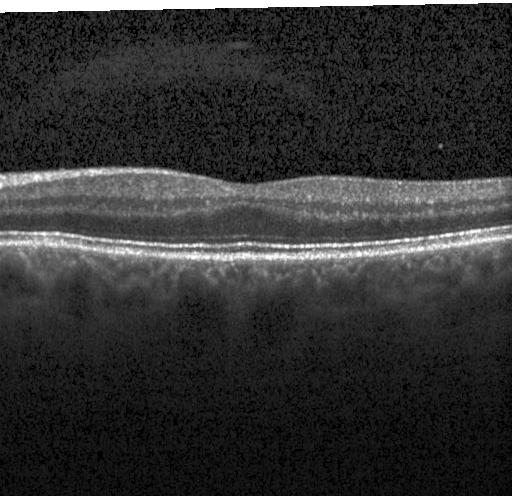
Spectral-domain OCT; Heidelberg Spectralis; optical coherence tomography B-scan — Dx: no CNV, no DME, and no drusen.